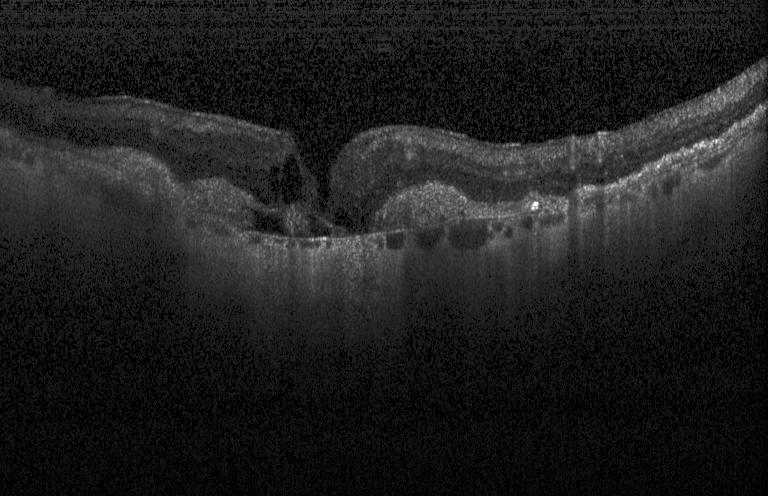
Finding: a choroidal neovascular membrane.